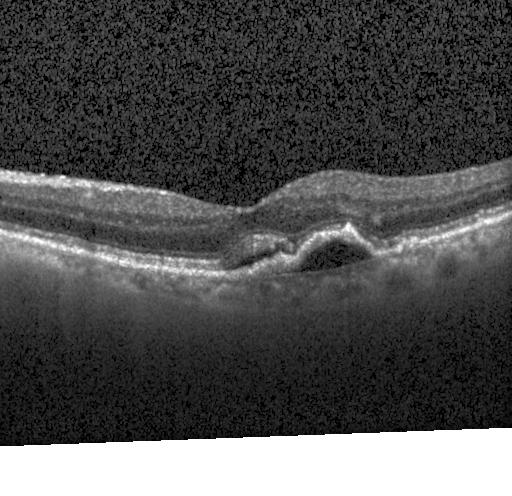
Dx: choroidal neovascularization.